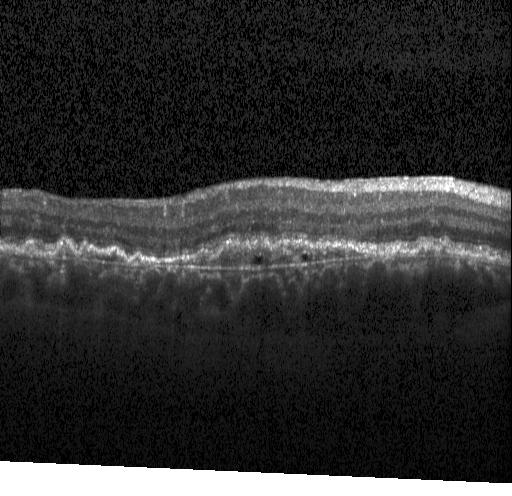

Optical coherence tomography scan — Macular OCT: choroidal neovascularization (CNV).